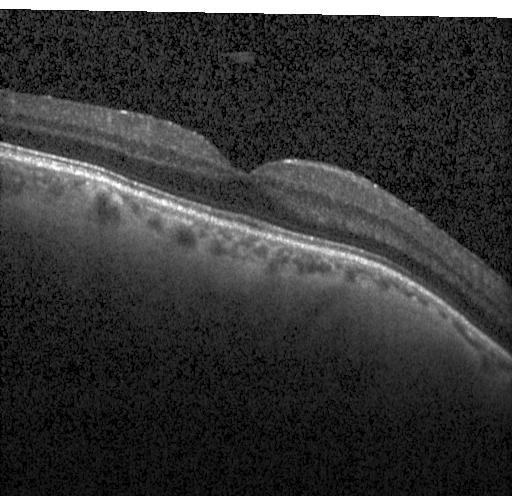

Heidelberg Spectralis · OCT B-scan · centered on the fovea · spectral-domain optical coherence tomography — No choroidal neovascularization, diabetic macular edema, or drusen.